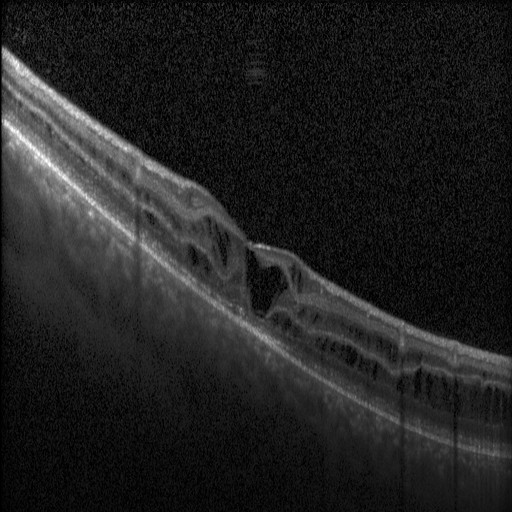 Retinal OCT B-scan.
Diagnosis: DME.